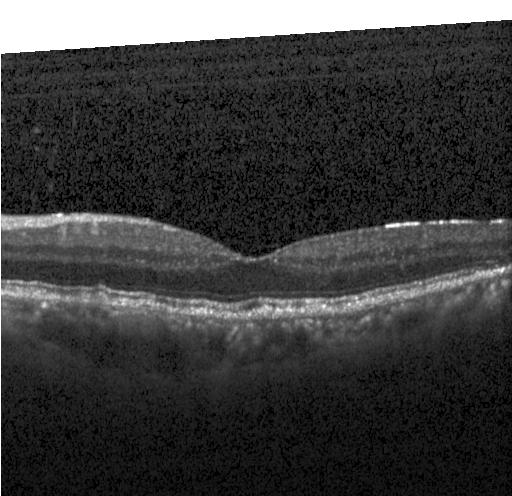
OCT scan showing multiple drusen.